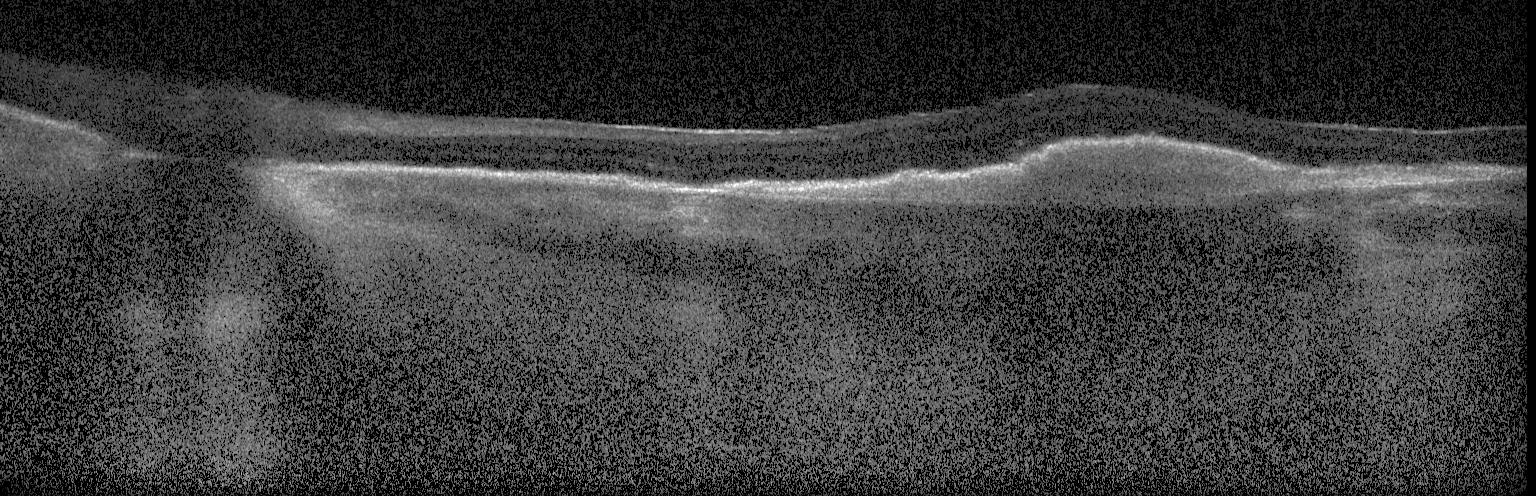
OCT B-scan
This B-scan demonstrates choroidal neovascularization (CNV).